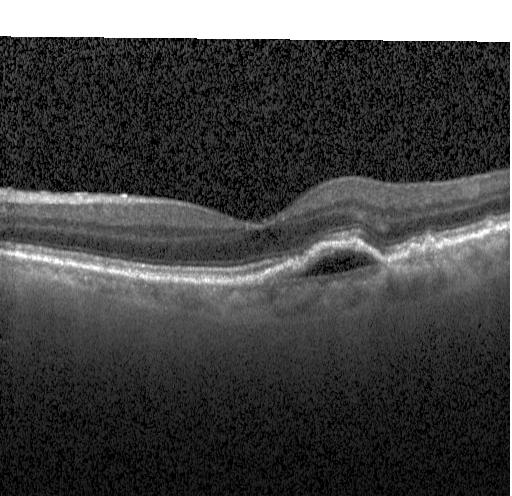
OCT line scan.
Finding: a choroidal neovascular membrane.